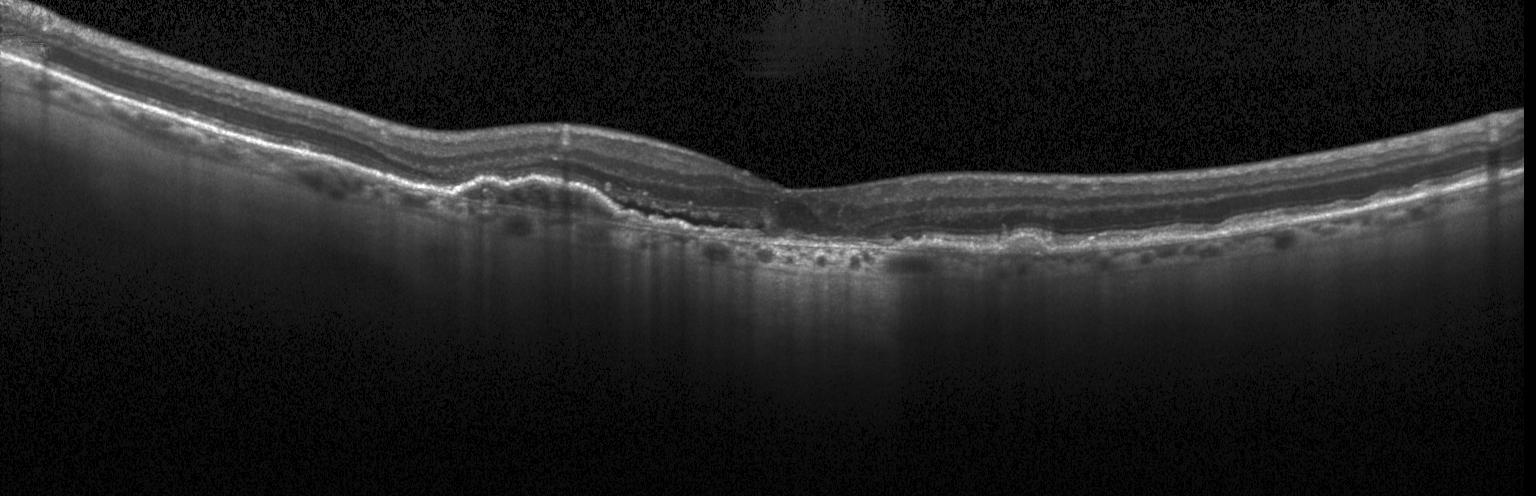 Impression: a choroidal neovascular membrane.